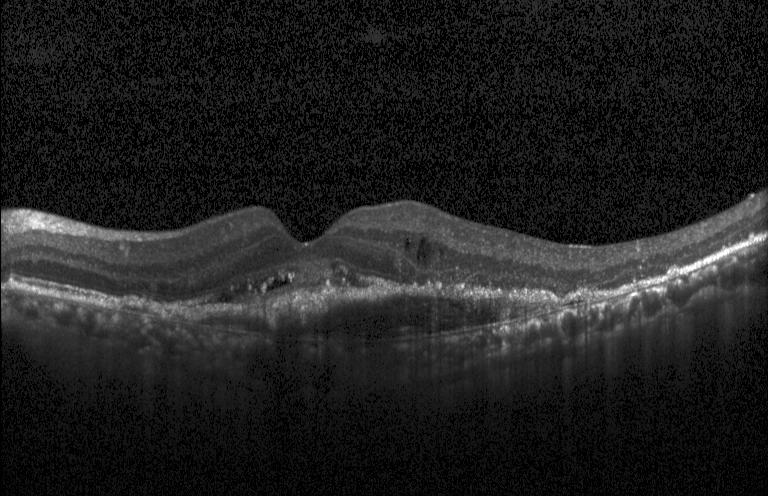

OCT line scan. Assessment: a choroidal neovascular membrane.